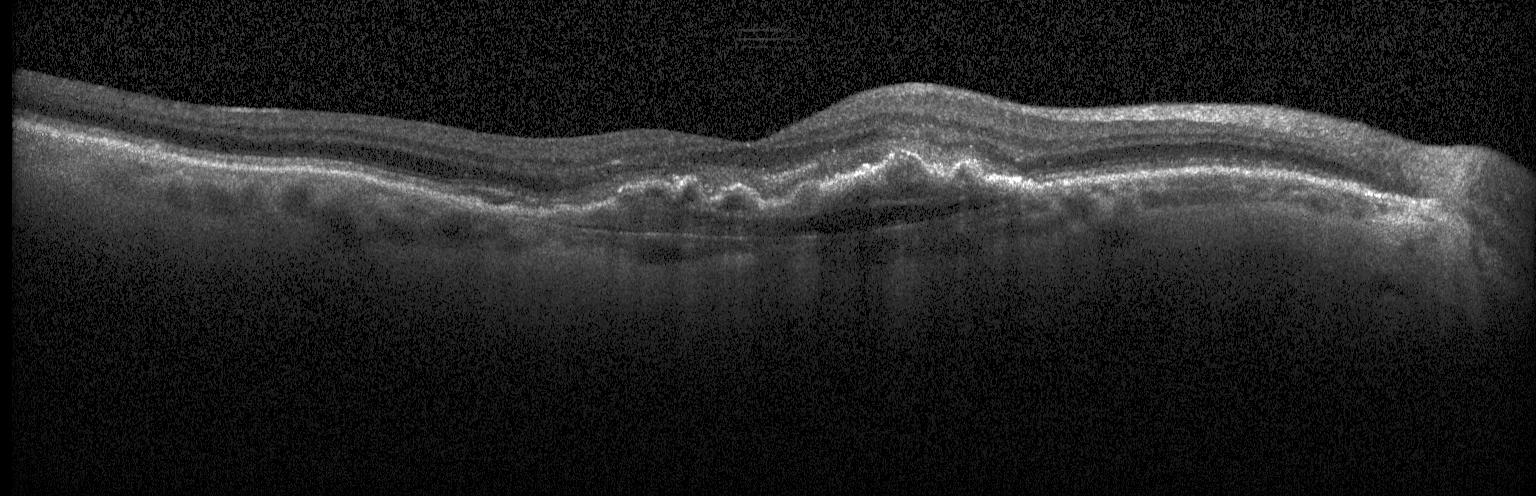 Optical coherence tomography scan · spectral-domain optical coherence tomography · acquired on a Heidelberg Spectralis
Macular OCT: a choroidal neovascular membrane.